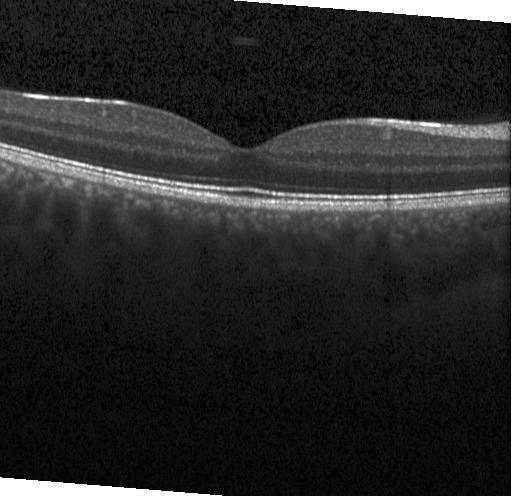 OCT B-scan
Macular OCT: no choroidal neovascularization, no diabetic macular edema, and no drusen.